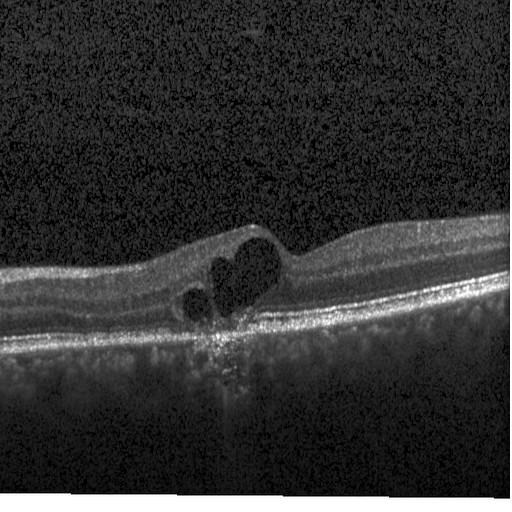

OCT B-scan, spectral-domain OCT, instrument: Heidelberg Spectralis.
Finding: diabetic macular edema (DME).